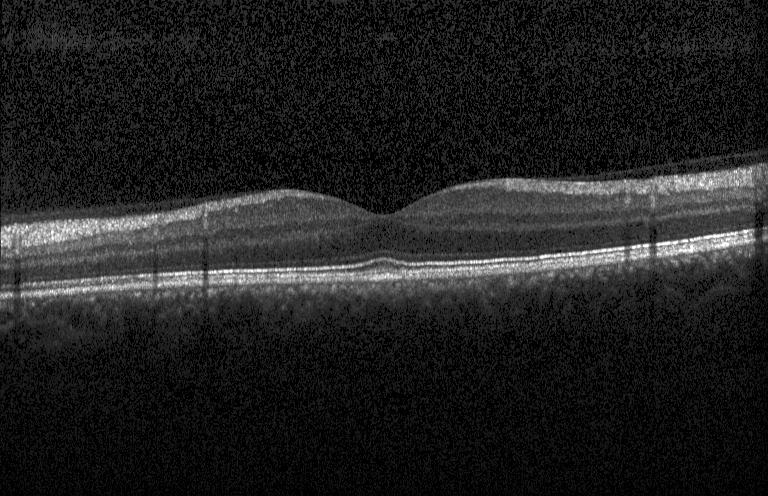 Optical coherence tomography scan · through the macula.
The scan shows no evidence of choroidal neovascularization, diabetic macular edema, or drusen.